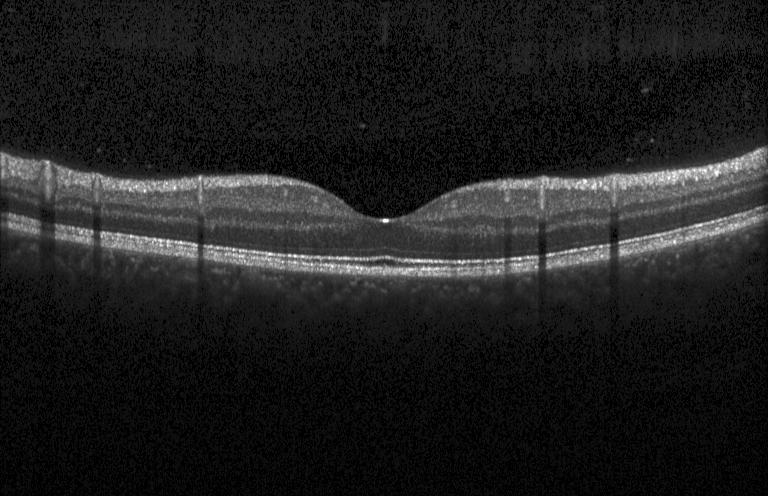
The scan shows no CNV, DME, or drusen.